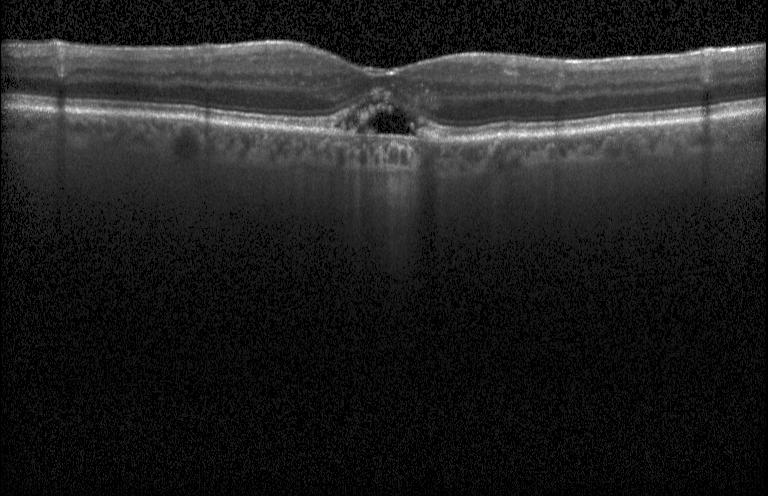
OCT line scan — Choroidal neovascularization (CNV).